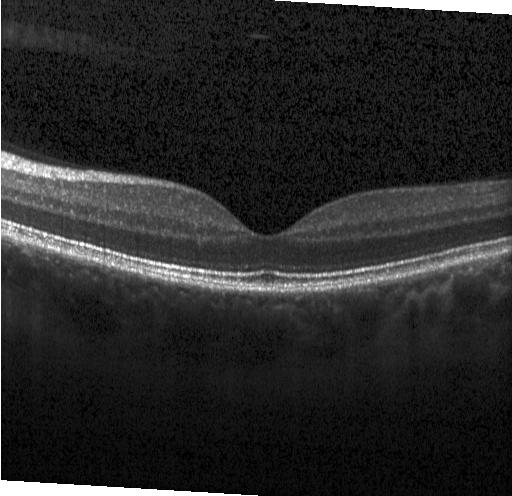

Optical coherence tomography scan. Spectral-domain OCT. Macular scan. Acquired on a Heidelberg Spectralis
The scan shows no choroidal neovascularization, no diabetic macular edema, and no drusen.